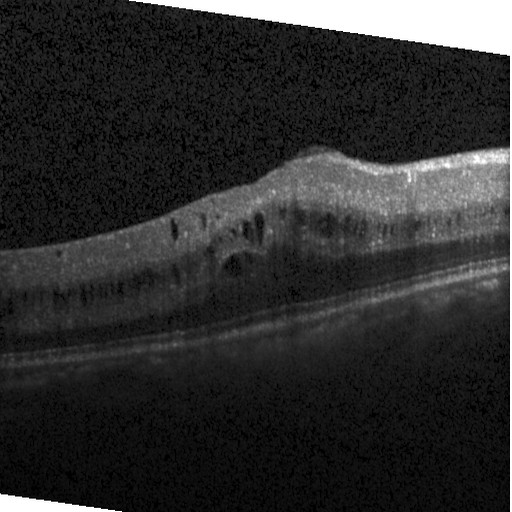 Impression: DME.